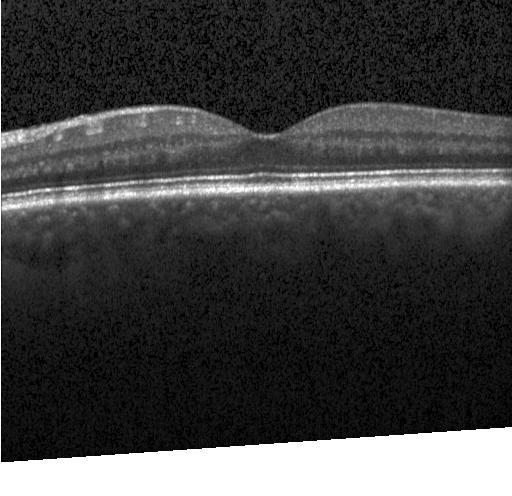
Spectral-domain OCT B-scan: neither choroidal neovascularization, diabetic macular edema, nor drusen.